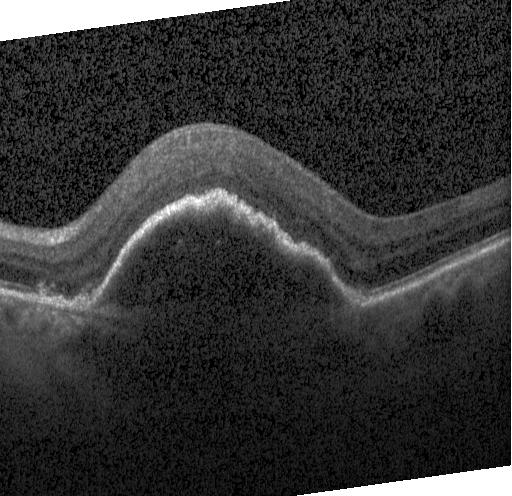 Diagnosis: a choroidal neovascular membrane.